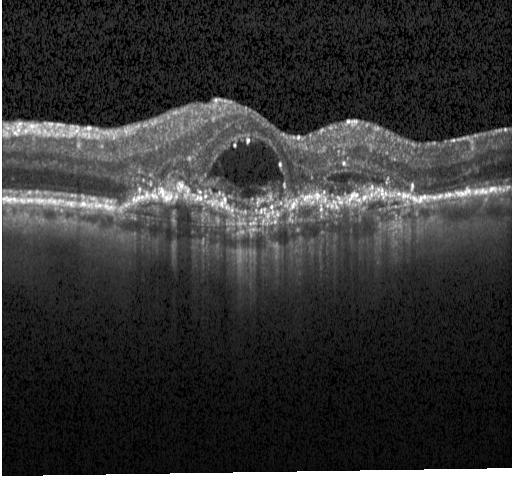
Impression: choroidal neovascularization.